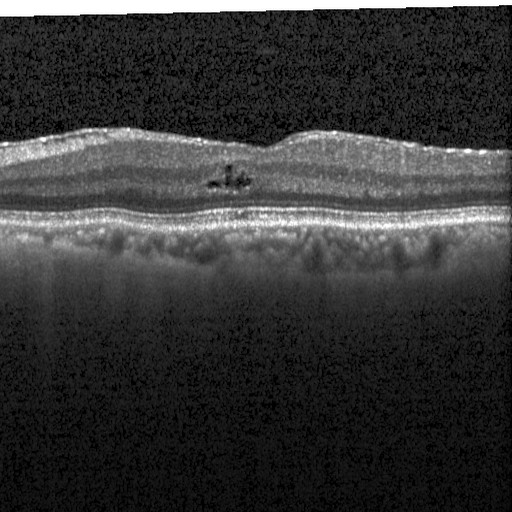

Spectral-domain OCT · Heidelberg Spectralis · centered on the fovea · OCT B-scan — OCT finding: DME.